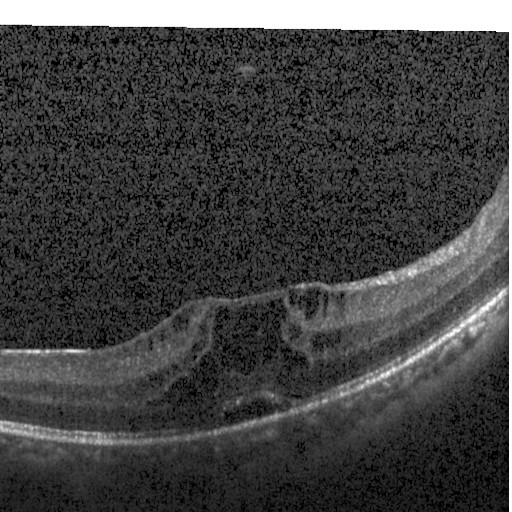 OCT scan showing diabetic macular edema (DME).